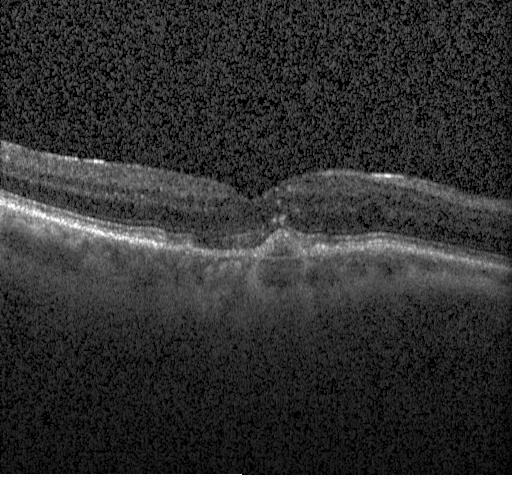

OCT line scan.
OCT finding: a choroidal neovascular membrane.